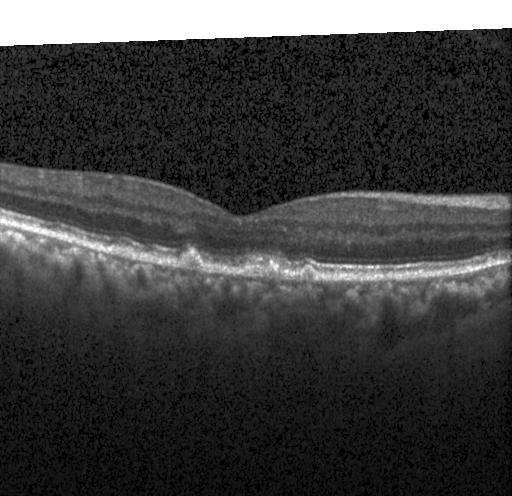
Diagnosis: multiple drusen.